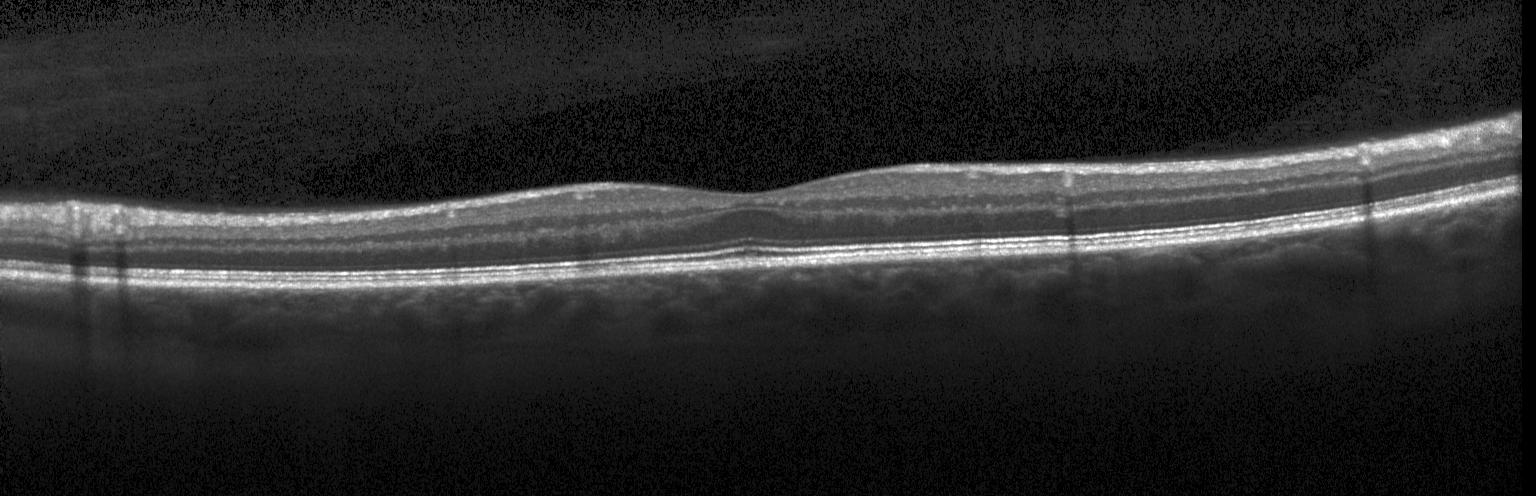 Instrument: Heidelberg Spectralis, spectral-domain OCT, centered on the fovea, optical coherence tomography B-scan — Finding: no choroidal neovascularization, no diabetic macular edema, and no drusen.